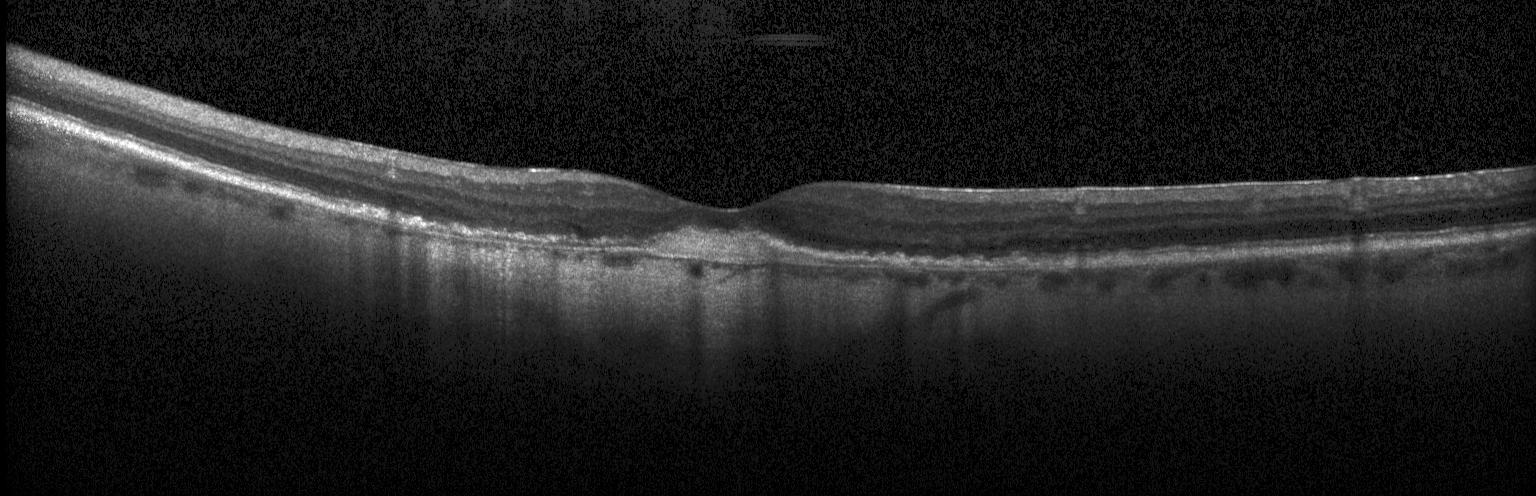

Spectral-domain optical coherence tomography; horizontal scan through the fovea; acquired on a Heidelberg Spectralis; optical coherence tomography B-scan. The scan shows choroidal neovascularization.